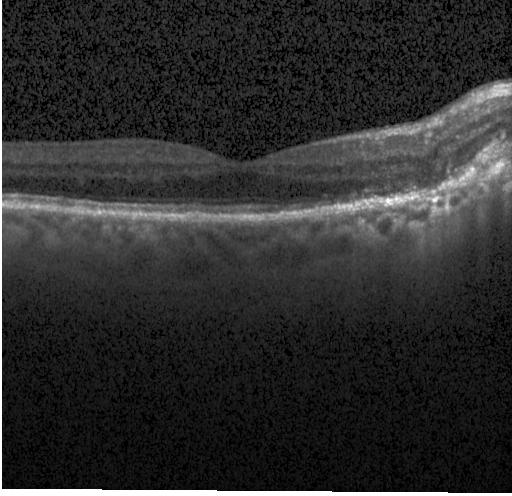
Instrument: Heidelberg Spectralis · optical coherence tomography scan
Finding: CNV.